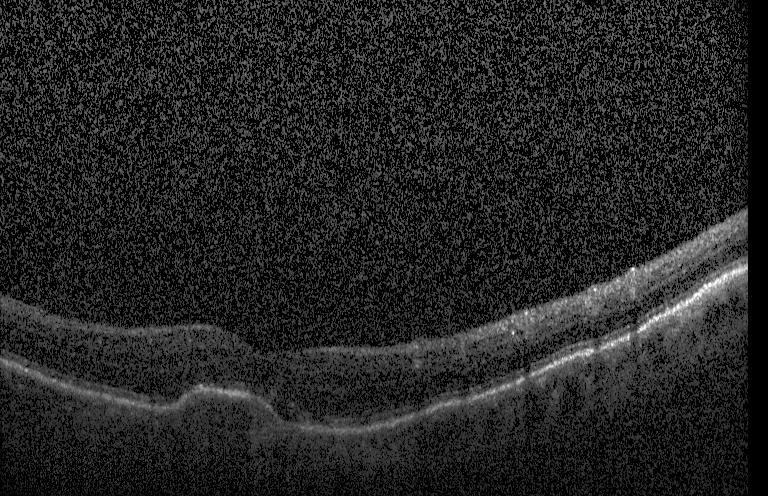

OCT scan showing a choroidal neovascular membrane.